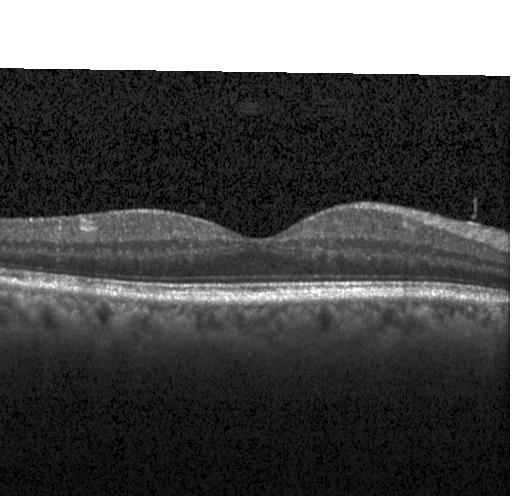 Dx: no choroidal neovascularization, diabetic macular edema, or drusen.